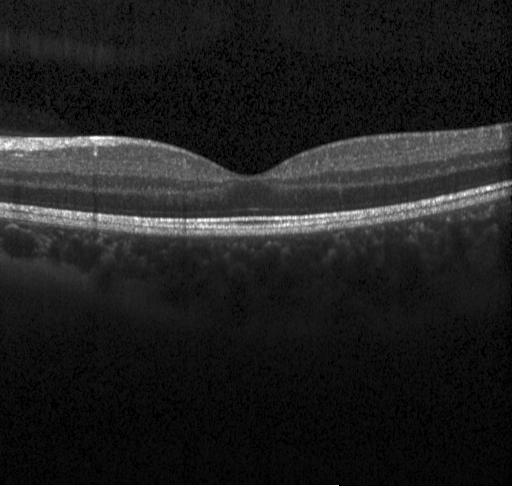

Optical coherence tomography B-scan; instrument: Heidelberg Spectralis; spectral-domain optical coherence tomography — Diagnosis: no evidence of choroidal neovascularization, diabetic macular edema, or drusen.